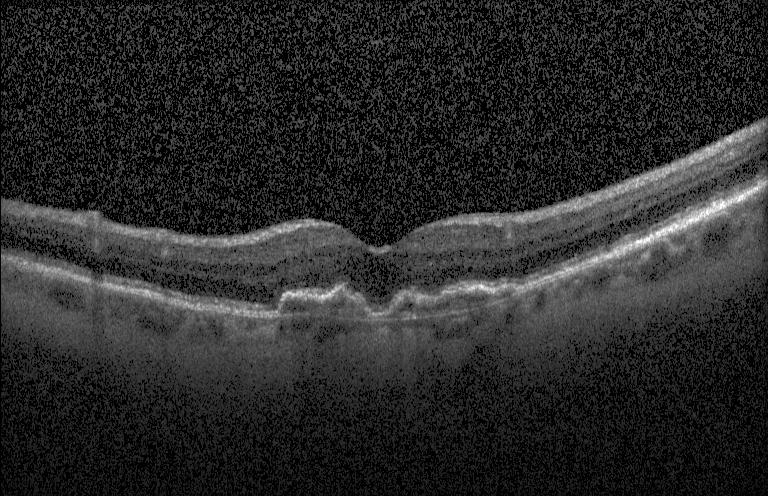 OCT line scan · centered on the fovea · acquired on a Heidelberg Spectralis.
Finding: a choroidal neovascular membrane.